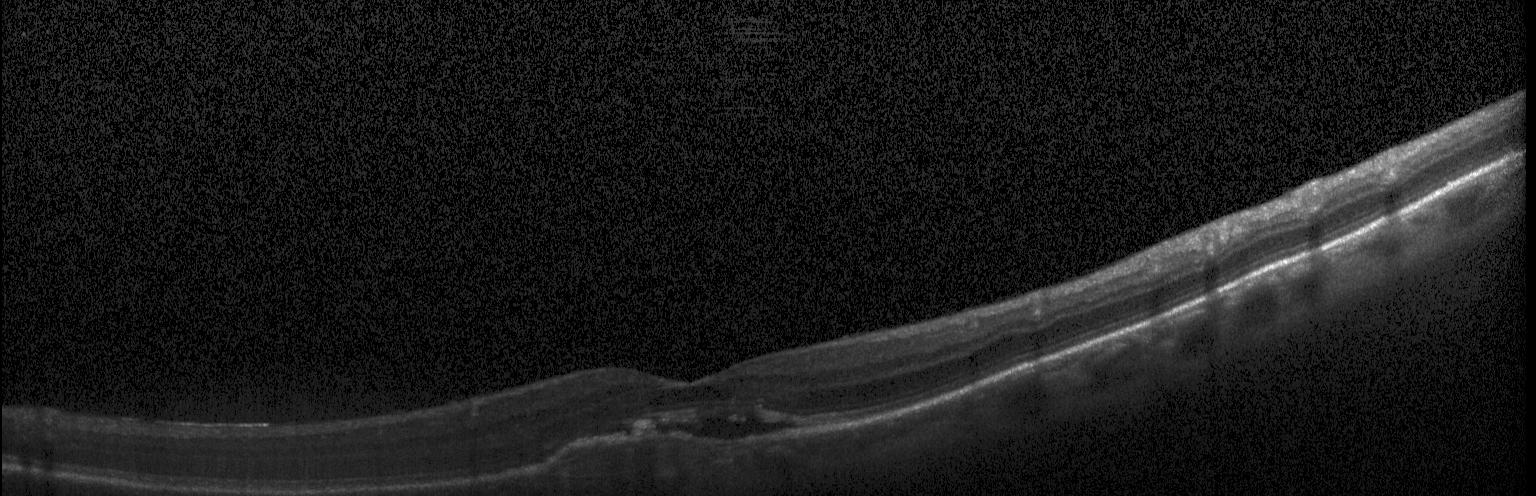 Horizontal scan through the fovea · OCT B-scan
Assessment: choroidal neovascularization (CNV).